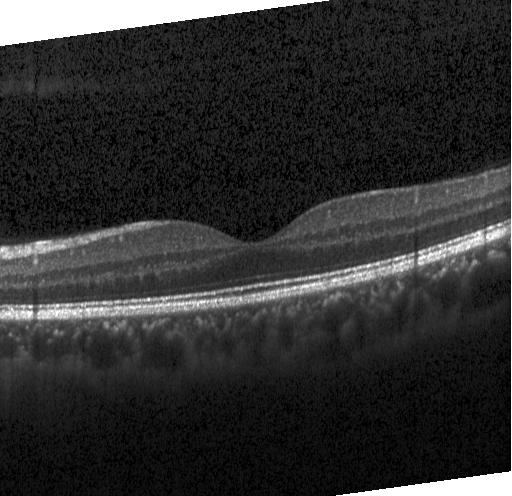 Macular scan; retinal OCT B-scan; Heidelberg Spectralis OCT system
The scan shows no choroidal neovascularization, diabetic macular edema, or drusen.